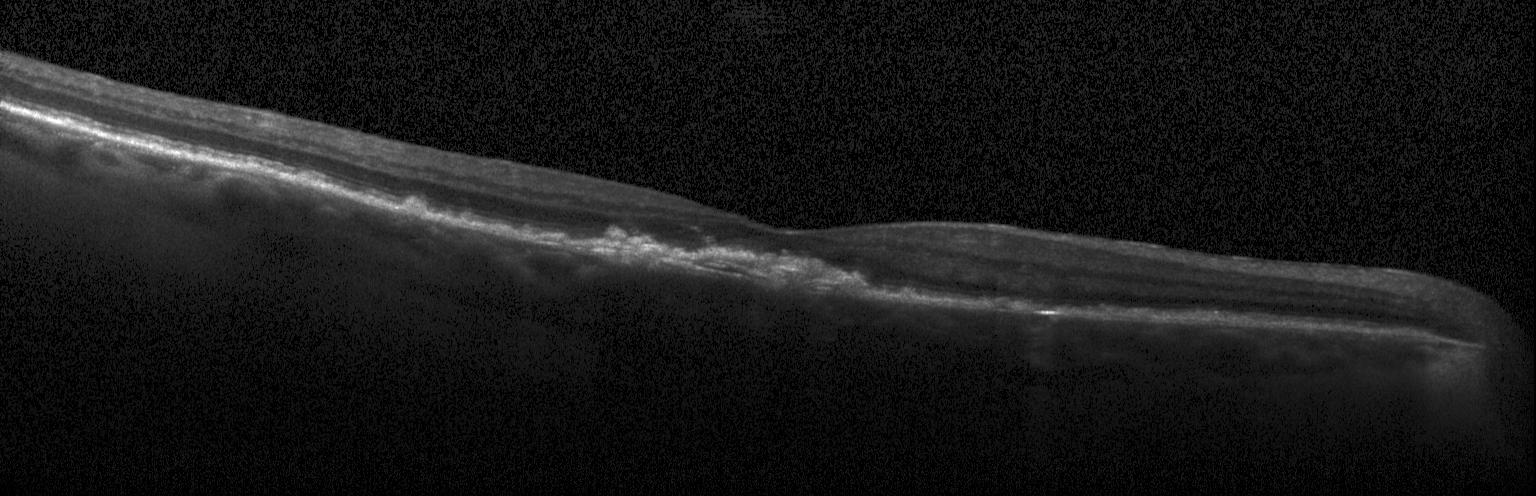
Optical coherence tomography scan; instrument: Heidelberg Spectralis; through the macula. OCT finding: a choroidal neovascular membrane.